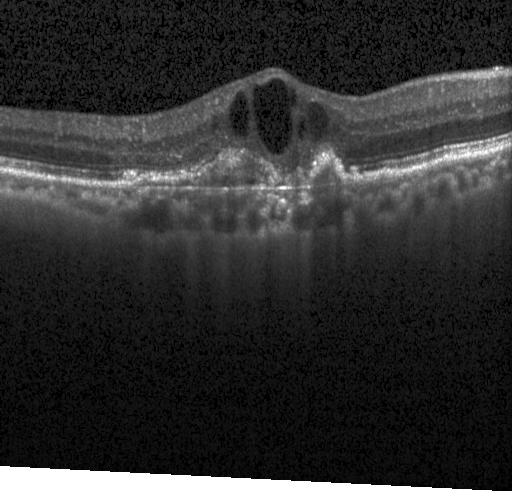
Horizontal scan through the fovea · OCT B-scan · acquired on a Heidelberg Spectralis.
Finding: a choroidal neovascular membrane.